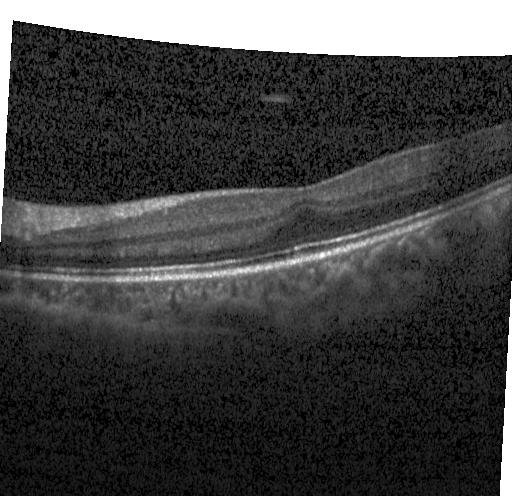
Retinal OCT B-scan.
No choroidal neovascularization, diabetic macular edema, or drusen.